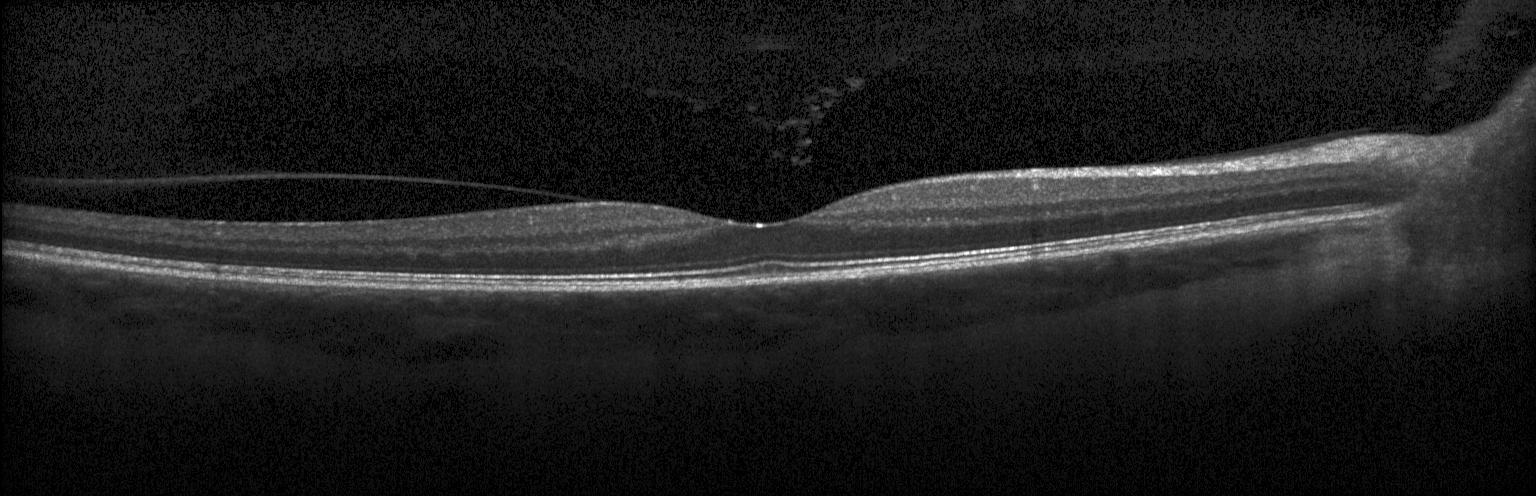 Spectral-domain OCT B-scan: no choroidal neovascularization, no diabetic macular edema, and no drusen.